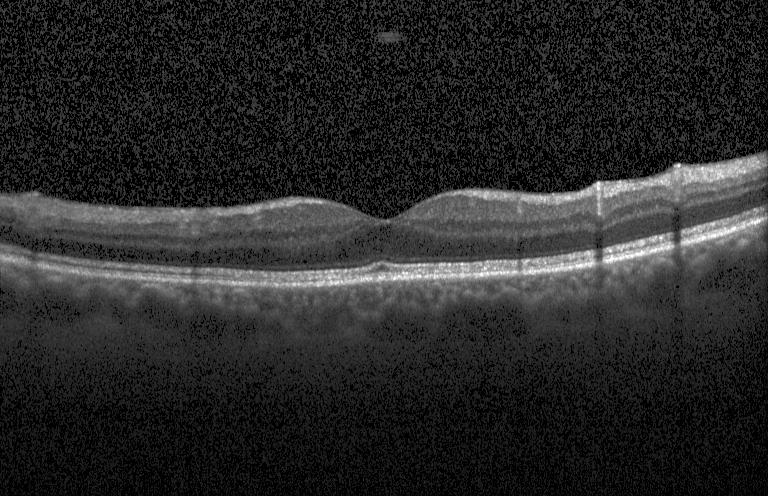 Impression: no choroidal neovascularization, diabetic macular edema, or drusen.